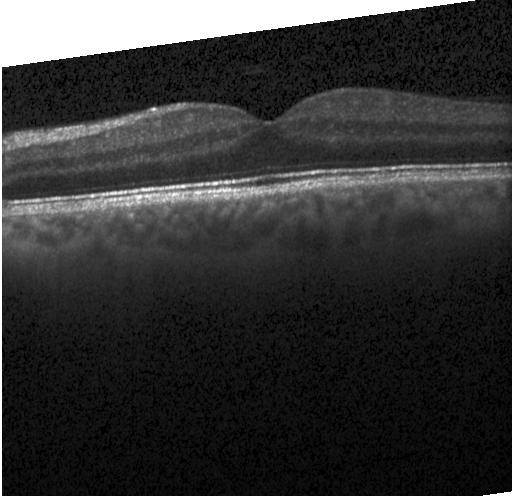
SD-OCT; retinal OCT B-scan.
Diagnosis: neither choroidal neovascularization, diabetic macular edema, nor drusen.